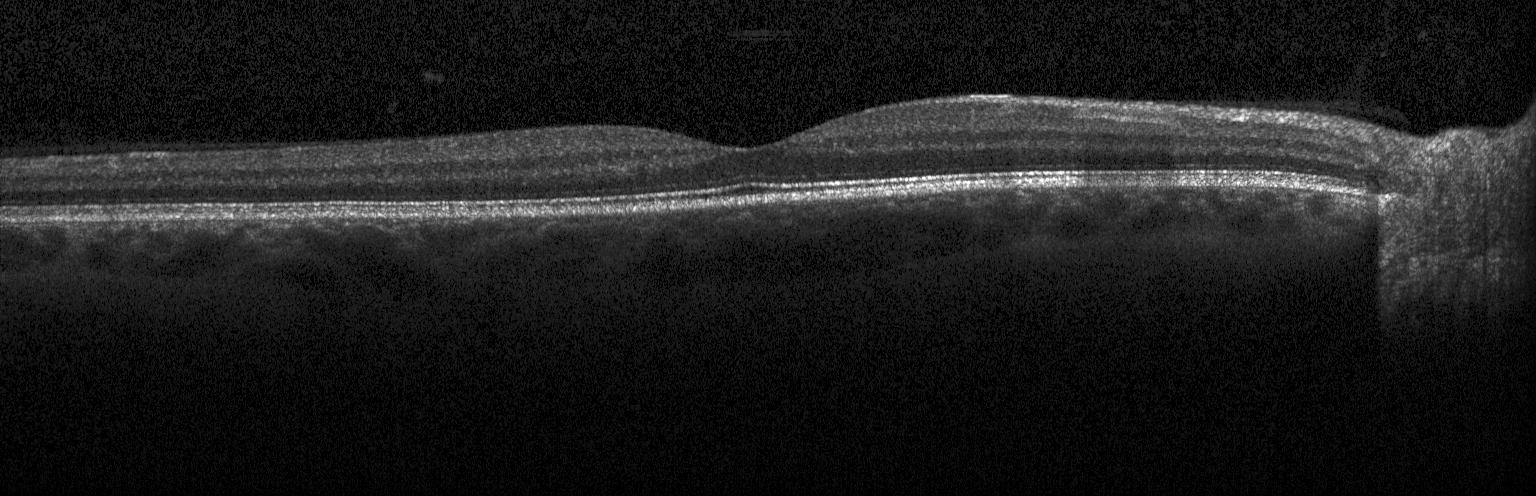
Instrument: Heidelberg Spectralis, retinal OCT cross-section, fovea-centered — No evidence of CNV, DME, or drusen.